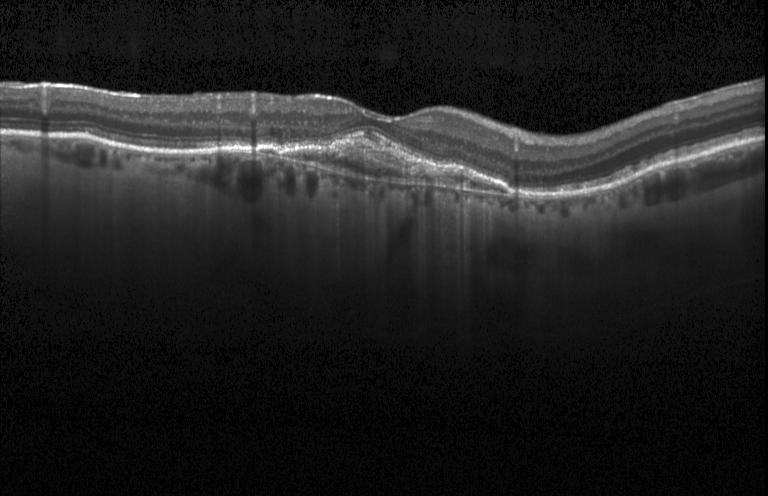
Finding: a choroidal neovascular membrane.